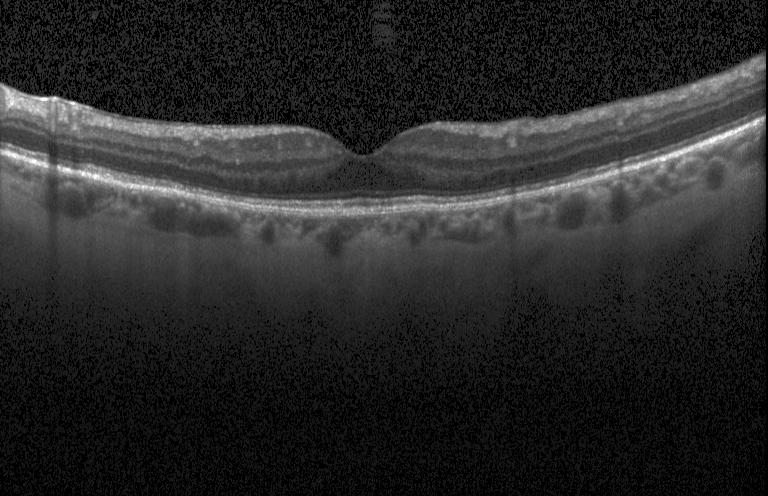

Optical coherence tomography scan. Acquired on a Heidelberg Spectralis. Spectral-domain optical coherence tomography. Macular scan — No evidence of CNV, DME, or drusen.